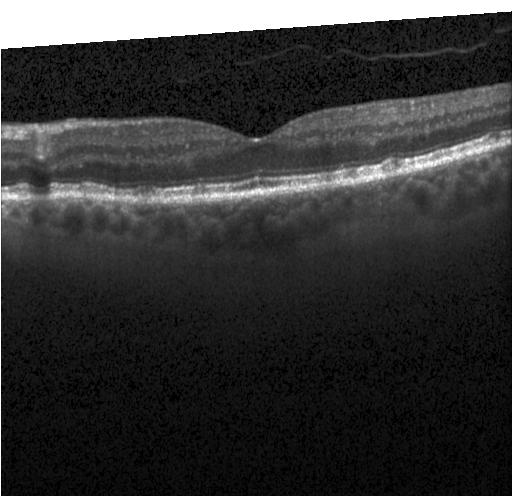

Retinal OCT B-scan. Spectral-domain optical coherence tomography. Diagnosis: drusen.